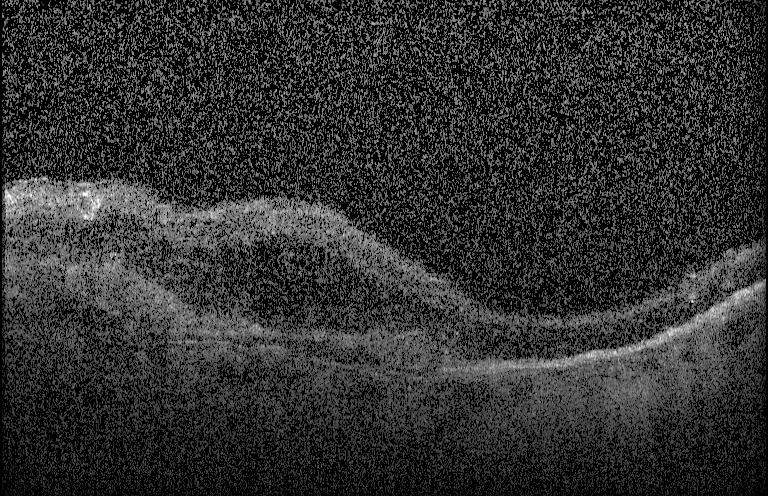

Instrument: Heidelberg Spectralis. Retinal OCT cross-section — Dx: CNV.